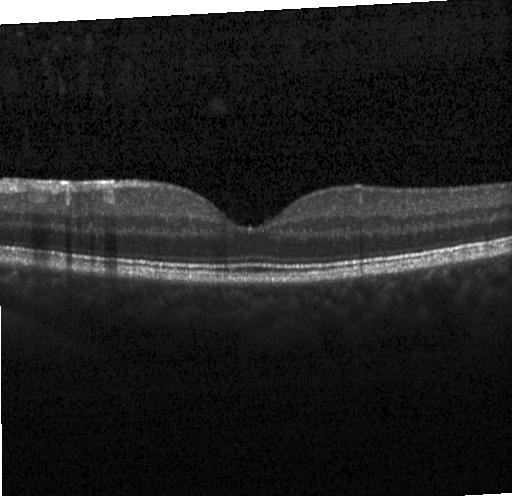
Optical coherence tomography B-scan · spectral-domain OCT
Impression: no choroidal neovascularization, no diabetic macular edema, and no drusen.